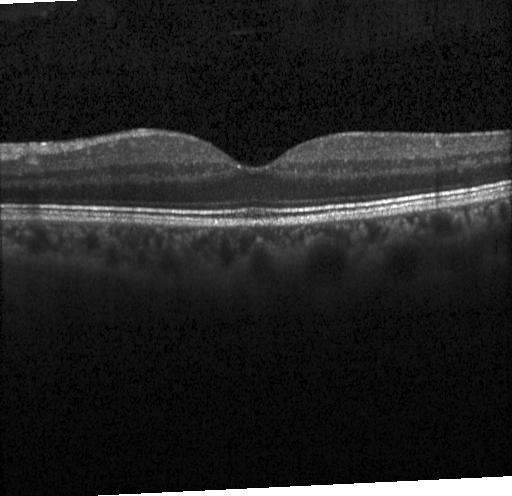

Instrument: Heidelberg Spectralis, spectral-domain OCT, through the macula, OCT line scan — Impression: neither choroidal neovascularization, diabetic macular edema, nor drusen.